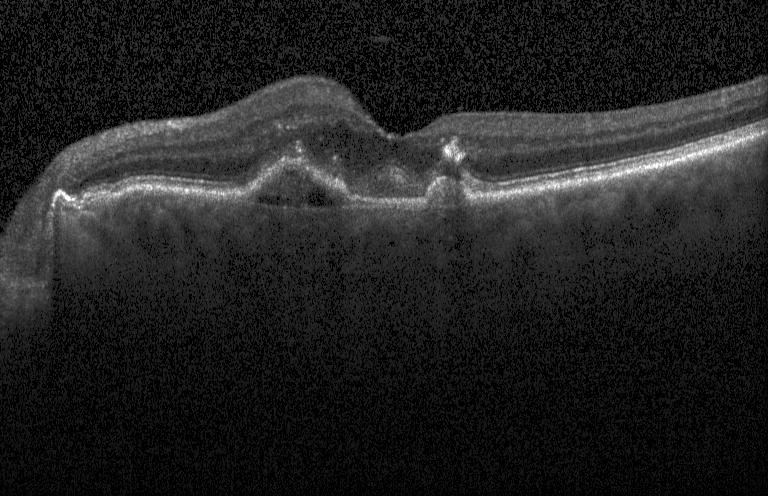
SD-OCT · centered on the fovea · OCT B-scan — Finding: a choroidal neovascular membrane.